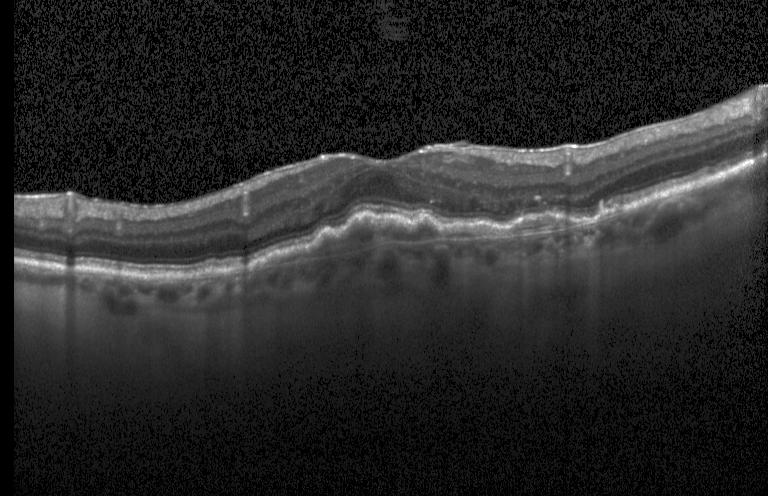

Diagnosis: choroidal neovascularization (CNV).